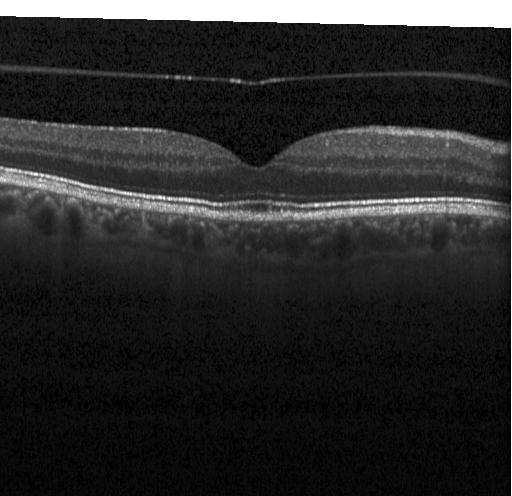

Assessment: neither CNV, DME, nor drusen.